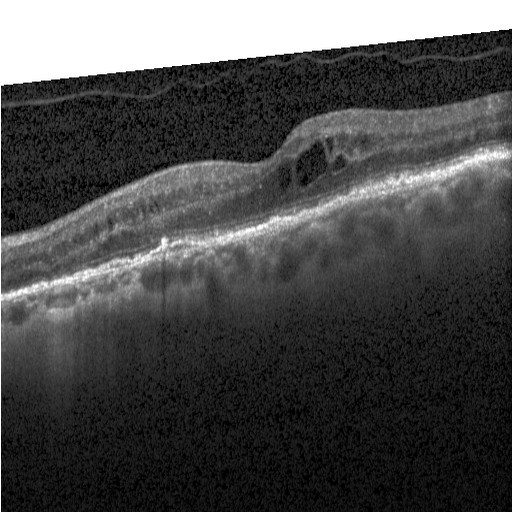
Spectral-domain optical coherence tomography · Heidelberg Spectralis OCT system · fovea-centered · OCT B-scan — Finding: DME.